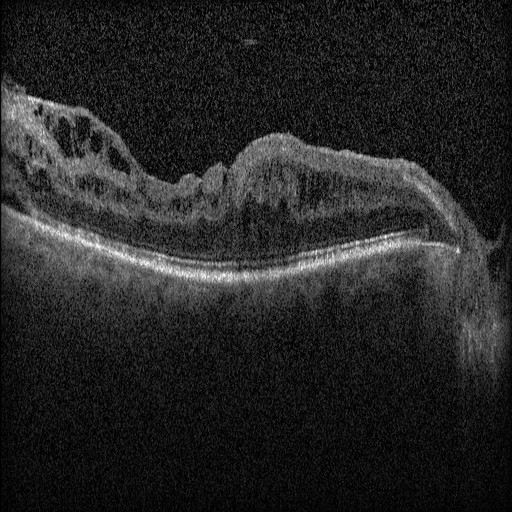

Heidelberg Spectralis OCT system; spectral-domain OCT; centered on the fovea; retinal OCT B-scan
Finding: DME.